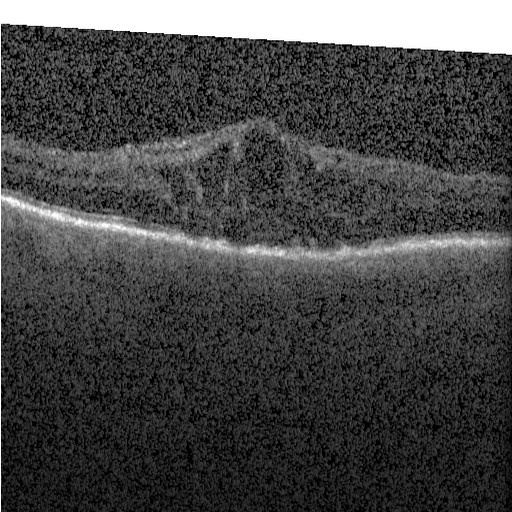

Heidelberg Spectralis · optical coherence tomography B-scan · horizontal scan through the fovea — Diagnosis: DME.